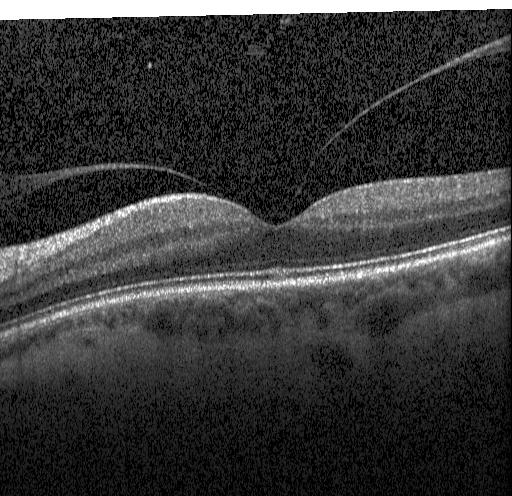 Diagnosis: no choroidal neovascularization, no diabetic macular edema, and no drusen.